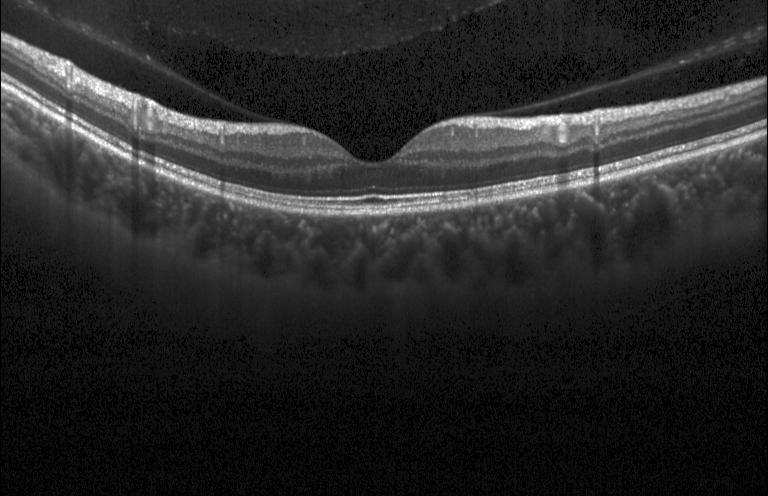

Assessment: no evidence of choroidal neovascularization, diabetic macular edema, or drusen.